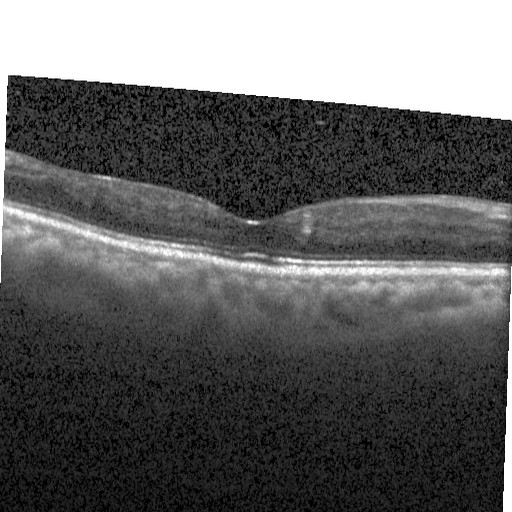 The scan shows diabetic macular edema.